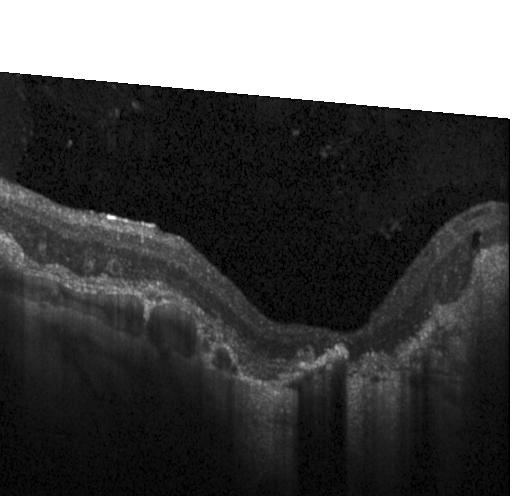 Spectral-domain OCT · optical coherence tomography scan · horizontal scan through the fovea · instrument: Heidelberg Spectralis — The scan shows a choroidal neovascular membrane.